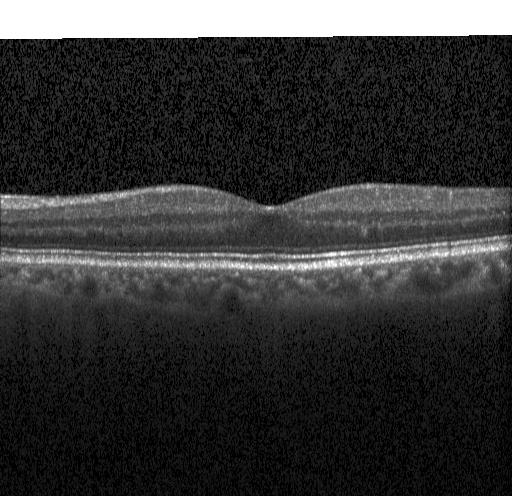
Retinal OCT B-scan.
No choroidal neovascularization, no diabetic macular edema, and no drusen.